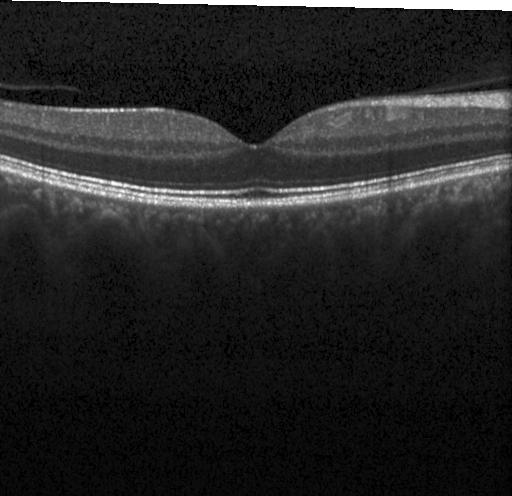 Macular OCT: neither choroidal neovascularization, diabetic macular edema, nor drusen.